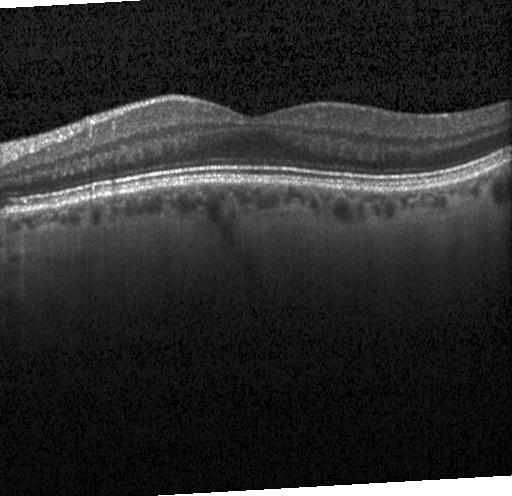
No choroidal neovascularization, diabetic macular edema, or drusen.